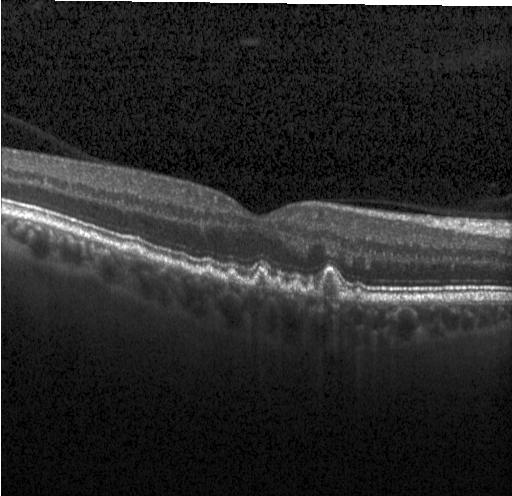

Macular OCT: multiple drusen.